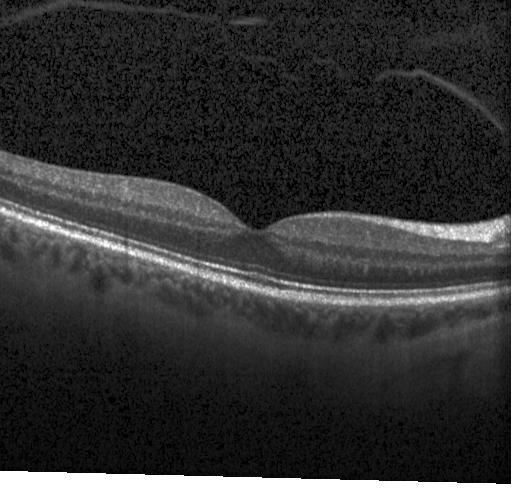 OCT B-scan
Finding: no CNV, no DME, and no drusen.